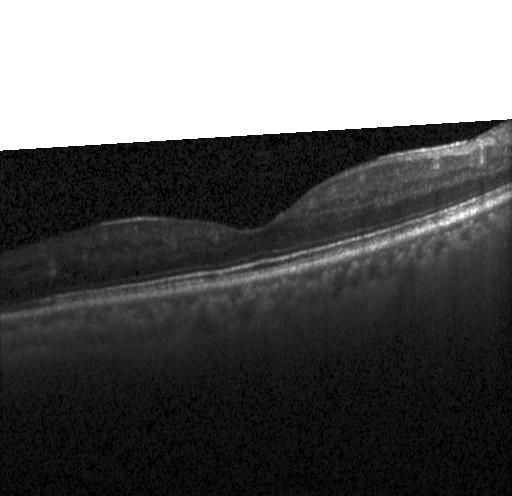 Retinal OCT B-scan; Heidelberg Spectralis; spectral-domain optical coherence tomography
Assessment: no CNV, DME, or drusen.